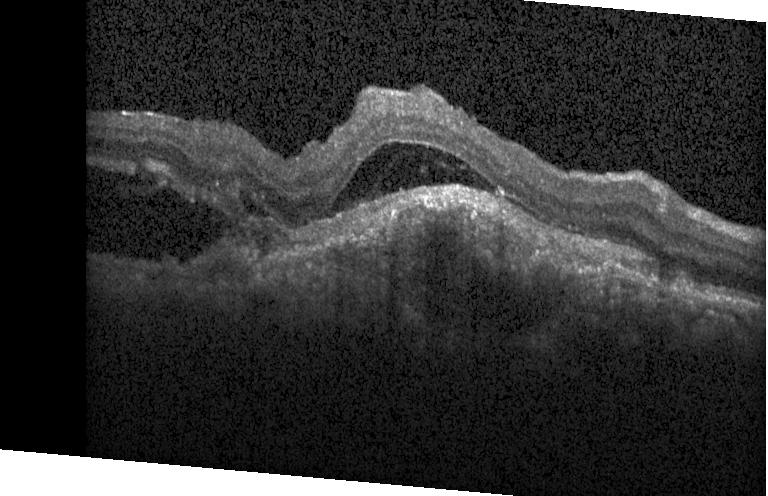
Instrument: Heidelberg Spectralis. OCT line scan — Macular OCT: a choroidal neovascular membrane.